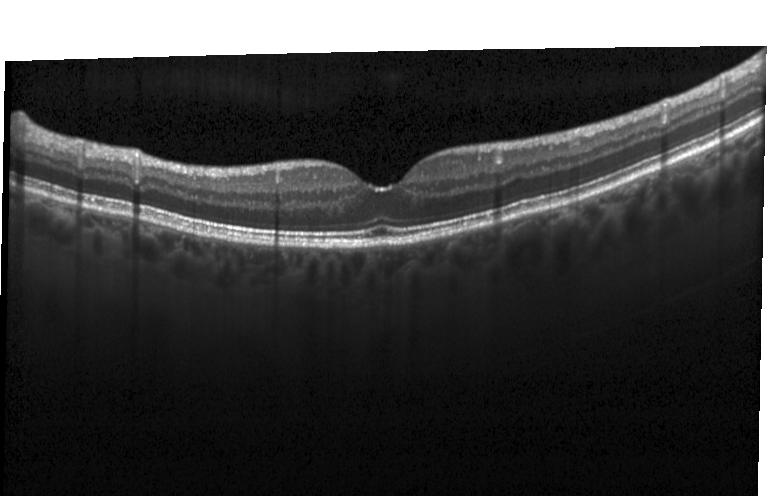
Dx: no choroidal neovascularization, diabetic macular edema, or drusen.